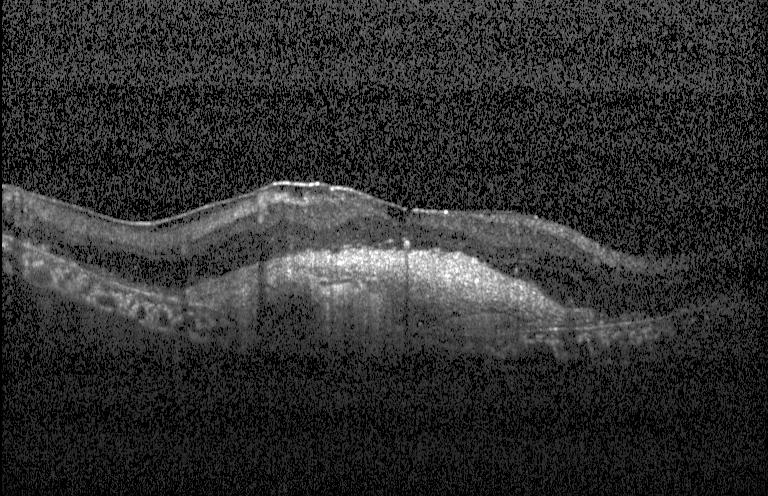
Diagnosis: a choroidal neovascular membrane.